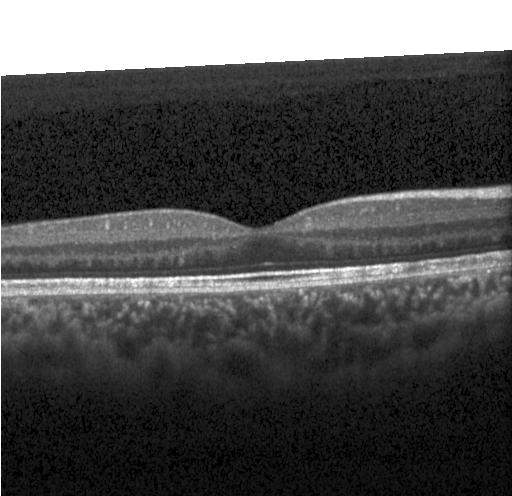

OCT line scan · SD-OCT · centered on the fovea · Heidelberg Spectralis OCT system.
Dx: no evidence of CNV, DME, or drusen.